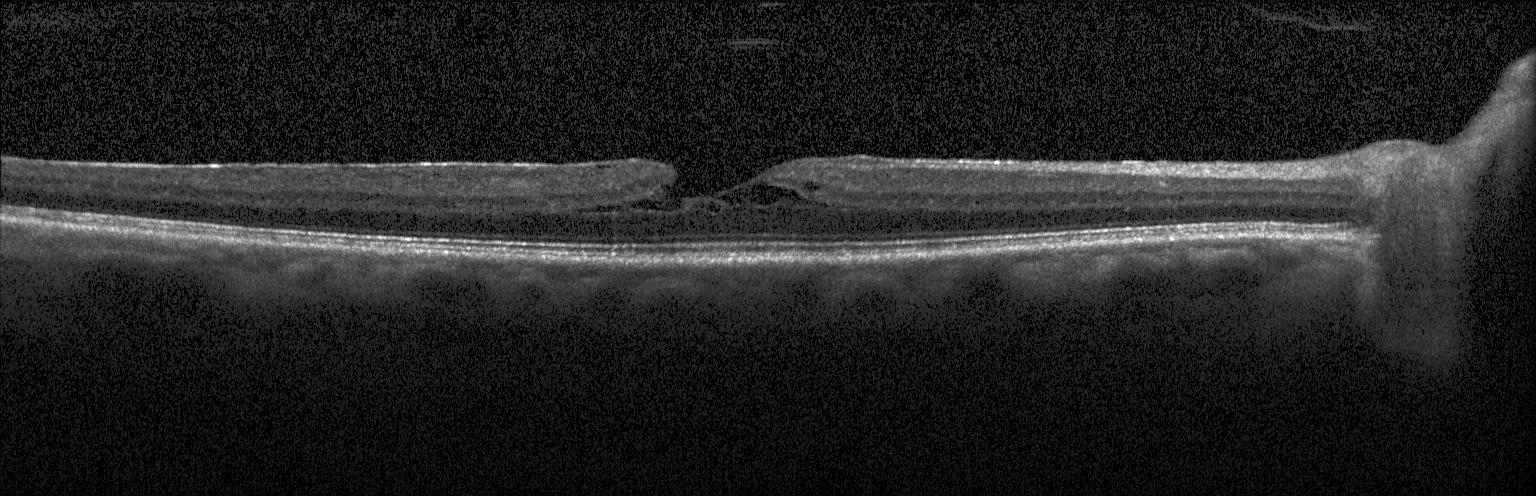 Centered on the fovea, optical coherence tomography B-scan.
The scan shows diabetic macular edema (DME).